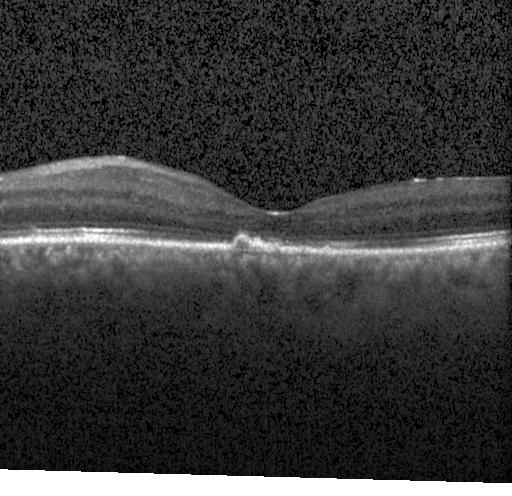
Heidelberg Spectralis. SD-OCT. OCT B-scan.
Impression: multiple drusen.